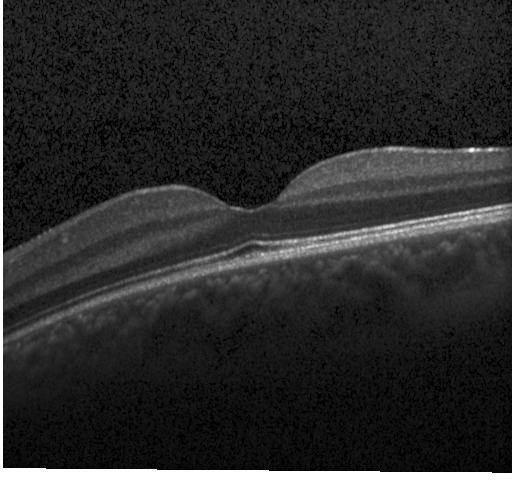
OCT line scan
Macular OCT: no choroidal neovascularization, no diabetic macular edema, and no drusen.